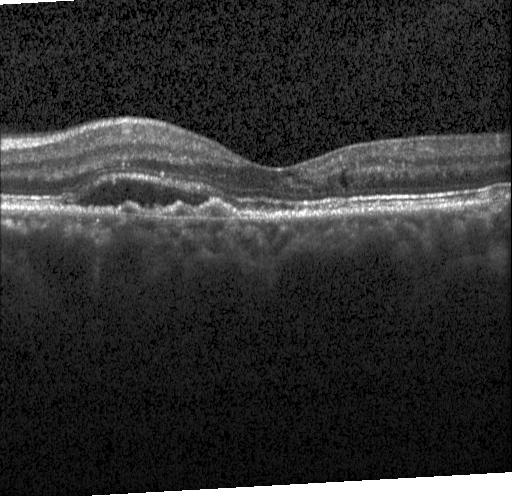
OCT scan showing CNV.